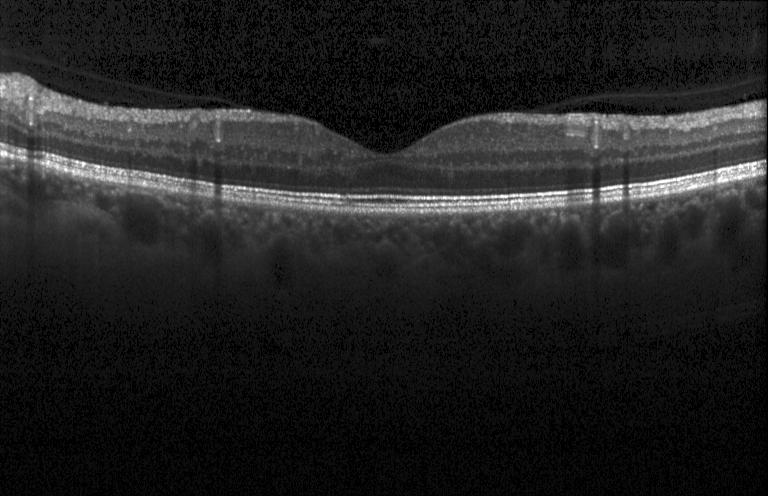 Spectral-domain optical coherence tomography; OCT line scan; through the macula — Finding: no choroidal neovascularization, no diabetic macular edema, and no drusen.